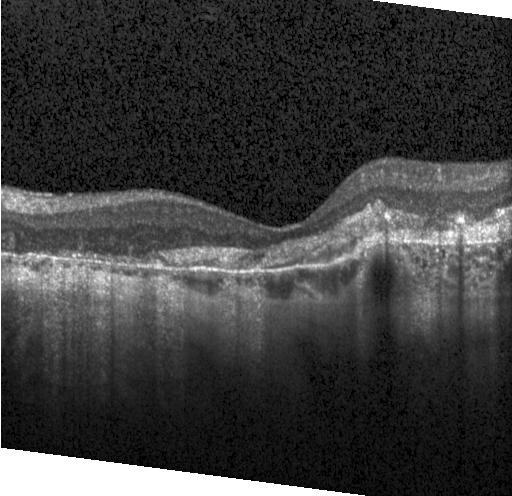
OCT B-scan — This B-scan demonstrates choroidal neovascularization.